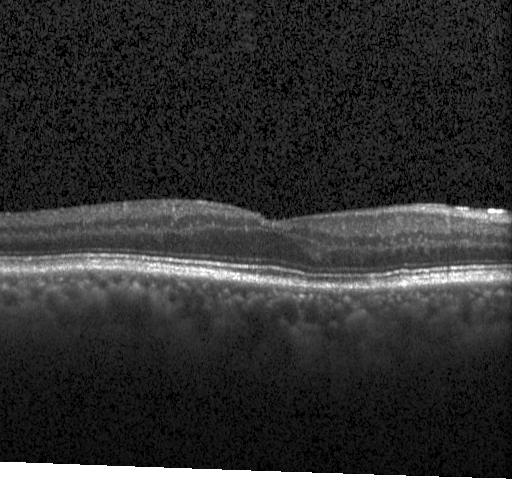 Diagnosis: no CNV, DME, or drusen.